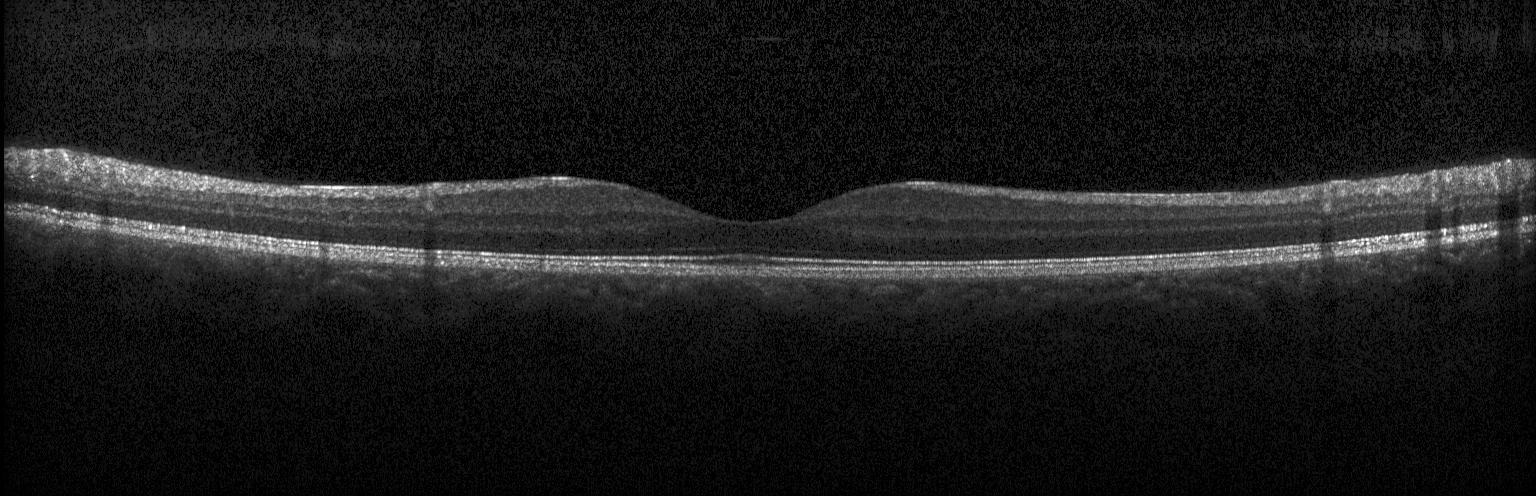 OCT B-scan.
Diagnosis: no evidence of CNV, DME, or drusen.